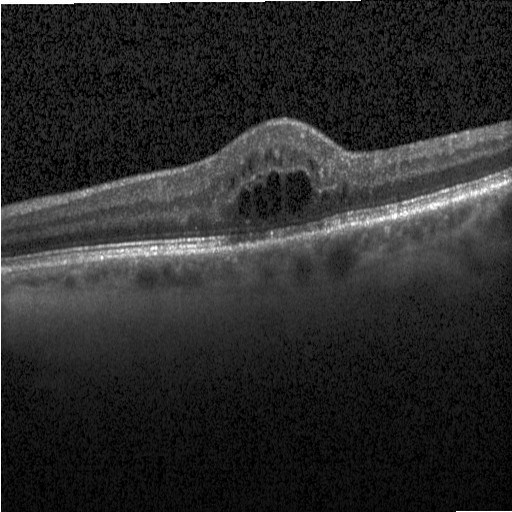 Optical coherence tomography B-scan, instrument: Heidelberg Spectralis, fovea-centered.
Impression: DME.